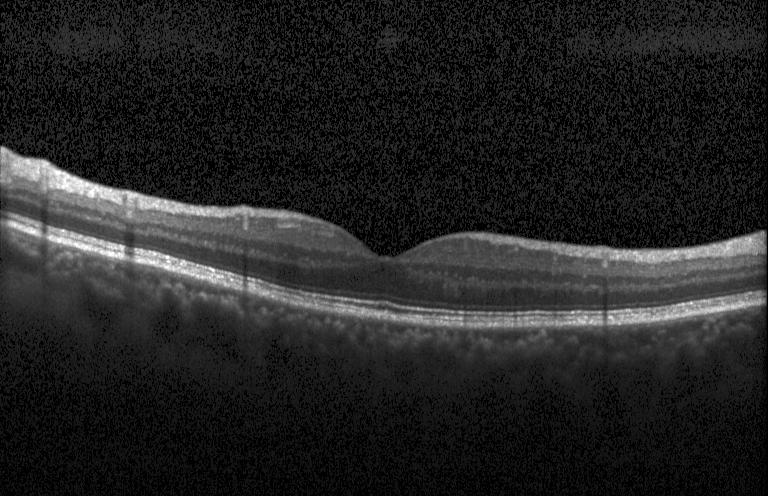
This B-scan demonstrates no evidence of choroidal neovascularization, diabetic macular edema, or drusen.